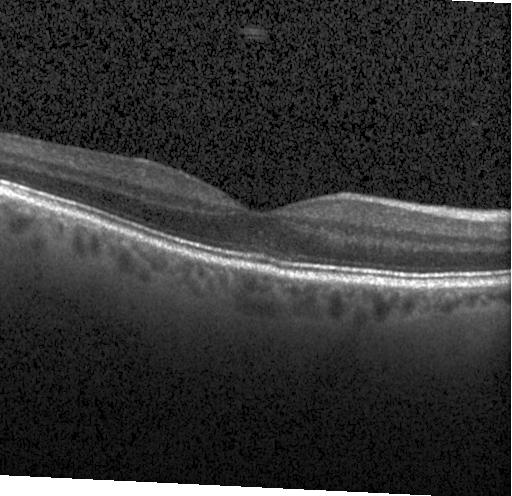
Optical coherence tomography scan · spectral-domain OCT.
Diagnosis: no choroidal neovascularization, no diabetic macular edema, and no drusen.